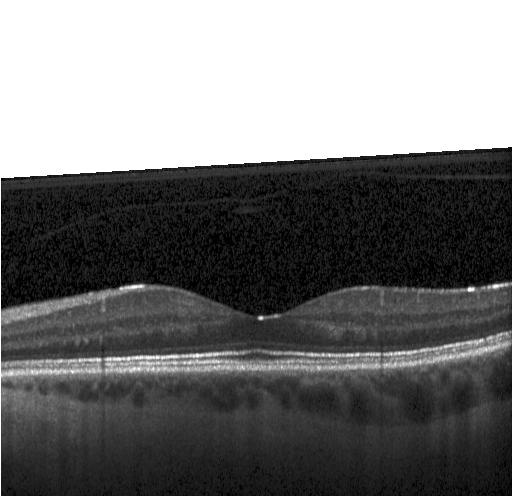
OCT line scan.
Finding: no choroidal neovascularization, no diabetic macular edema, and no drusen.